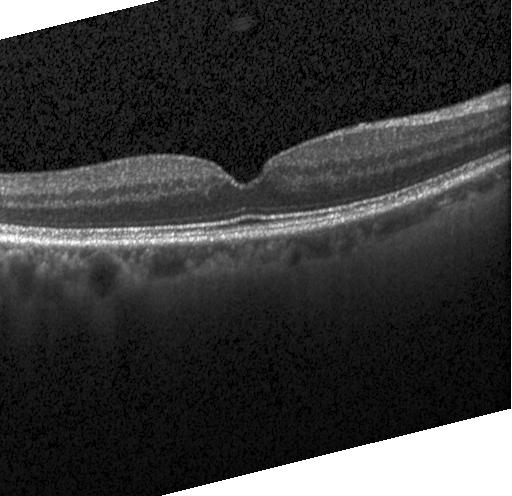 Through the macula. Spectral-domain OCT. Retinal OCT B-scan. Acquired on a Heidelberg Spectralis
Diagnosis: neither choroidal neovascularization, diabetic macular edema, nor drusen.